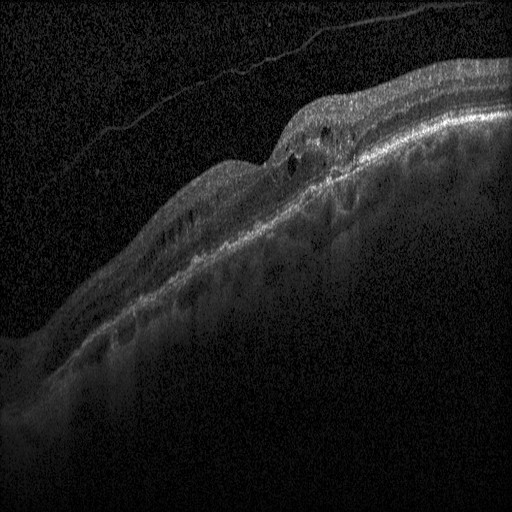
Spectral-domain optical coherence tomography; optical coherence tomography scan
Macular OCT: diabetic macular edema (DME).